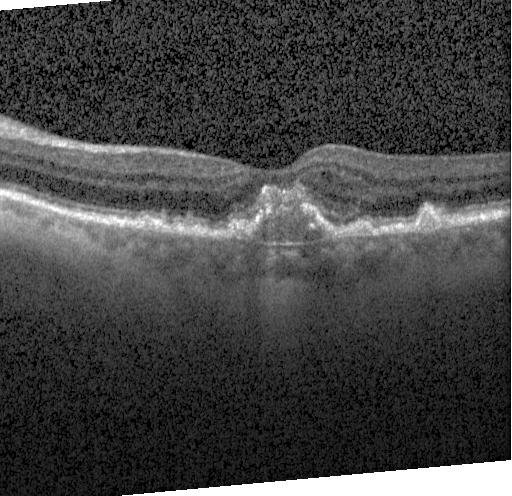

Centered on the fovea, spectral-domain OCT, retinal OCT cross-section. Macular OCT: choroidal neovascularization.